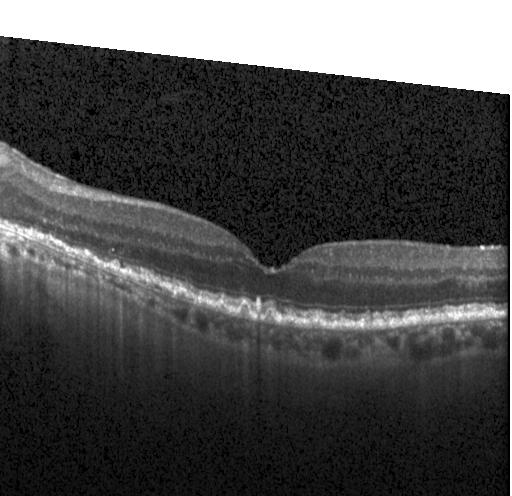
Acquired on a Heidelberg Spectralis · spectral-domain OCT · through the macula · retinal OCT cross-section. Diagnosis: sub-RPE drusenoid deposits.